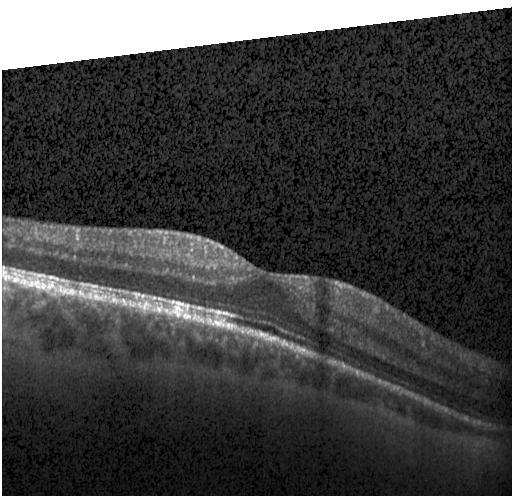 Heidelberg Spectralis OCT system; OCT line scan; SD-OCT. Finding: no evidence of choroidal neovascularization, diabetic macular edema, or drusen.